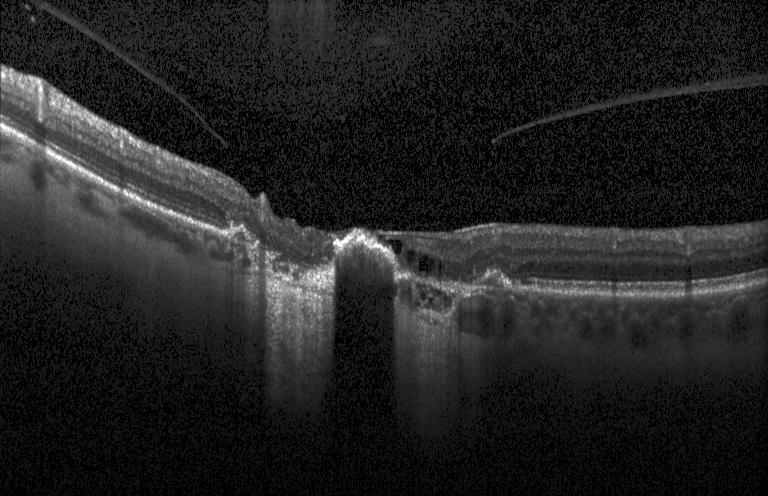

OCT line scan · instrument: Heidelberg Spectralis · SD-OCT · horizontal scan through the fovea. Dx: CNV.